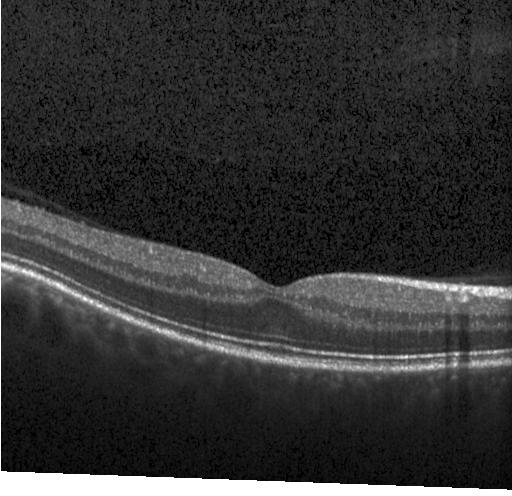

Retinal OCT B-scan · spectral-domain optical coherence tomography · Heidelberg Spectralis · macular scan
Diagnosis: no evidence of CNV, DME, or drusen.